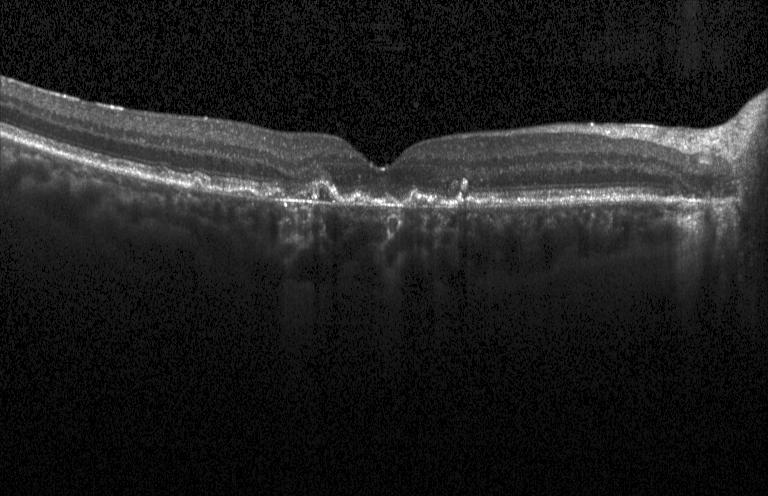
Through the macula. Retinal OCT B-scan. Acquired on a Heidelberg Spectralis — Diagnosis: a choroidal neovascular membrane.